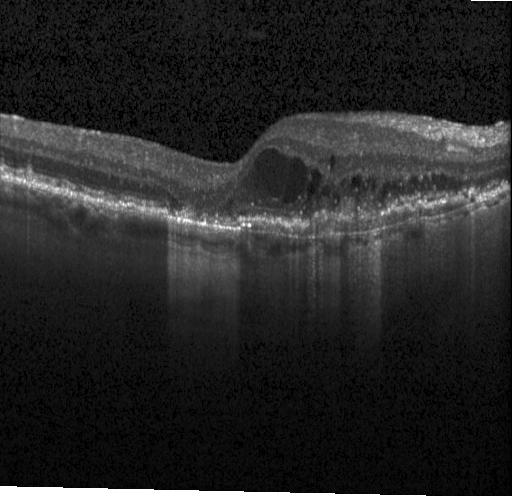 Heidelberg Spectralis · retinal OCT cross-section. OCT finding: choroidal neovascularization (CNV).